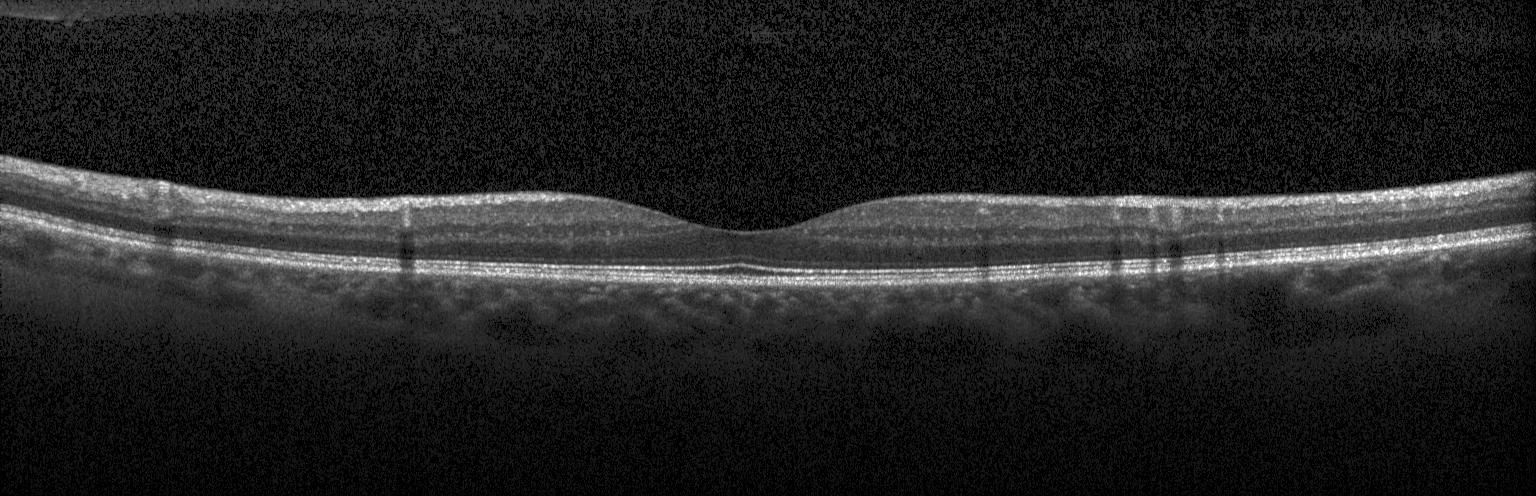 OCT line scan. Heidelberg Spectralis OCT system. The scan shows no choroidal neovascularization, diabetic macular edema, or drusen.